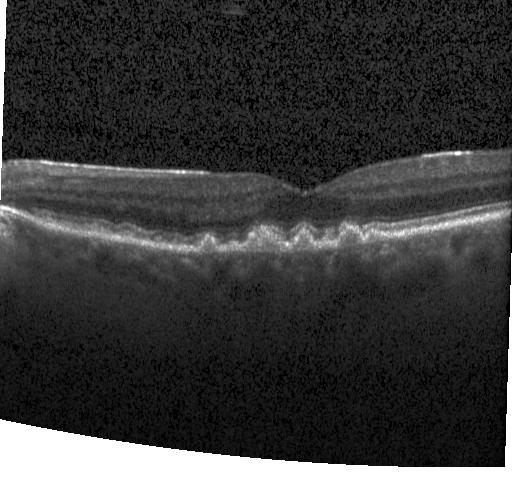

Dx: multiple drusen.